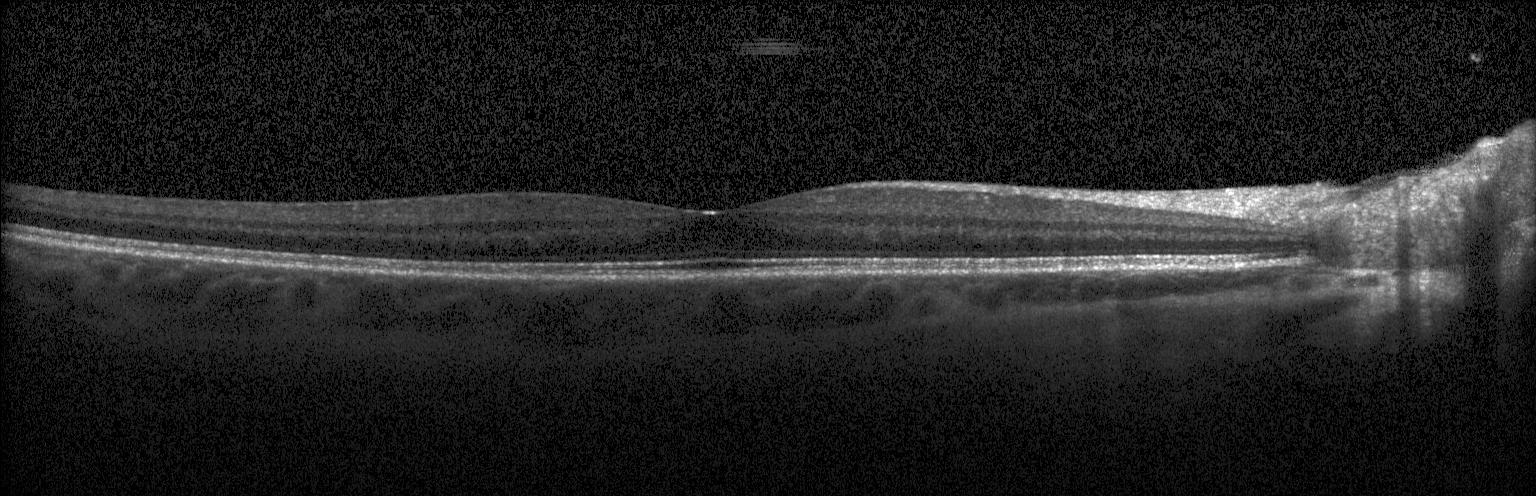 No evidence of choroidal neovascularization, diabetic macular edema, or drusen.